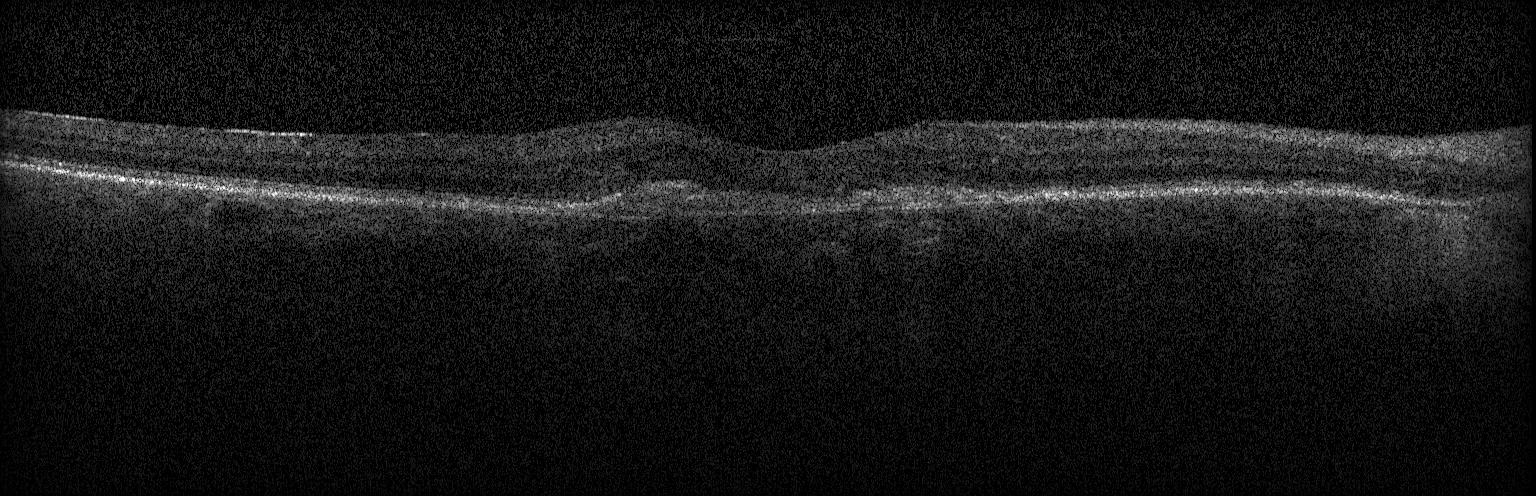

Macular OCT: a choroidal neovascular membrane.